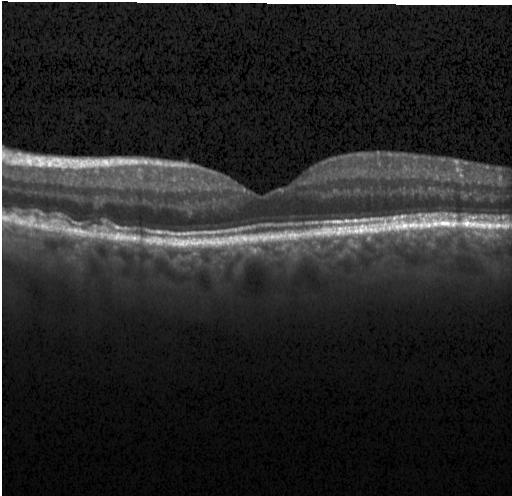

OCT B-scan; Heidelberg Spectralis OCT system; horizontal scan through the fovea
The scan shows drusen.